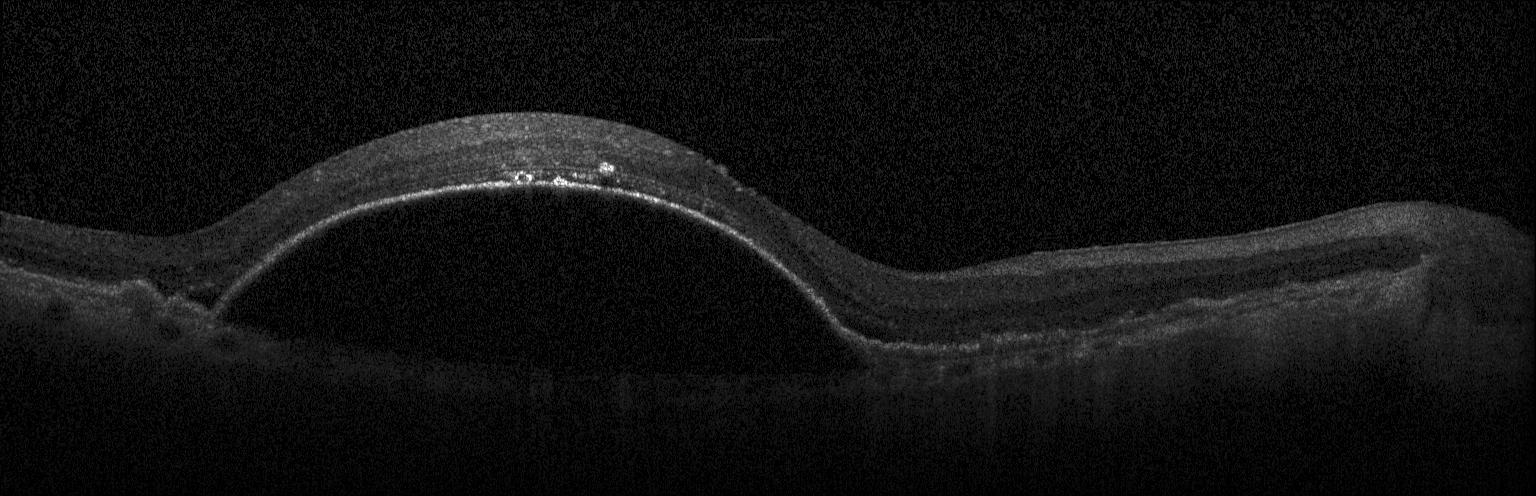 Retinal OCT cross-section.
Impression: CNV.